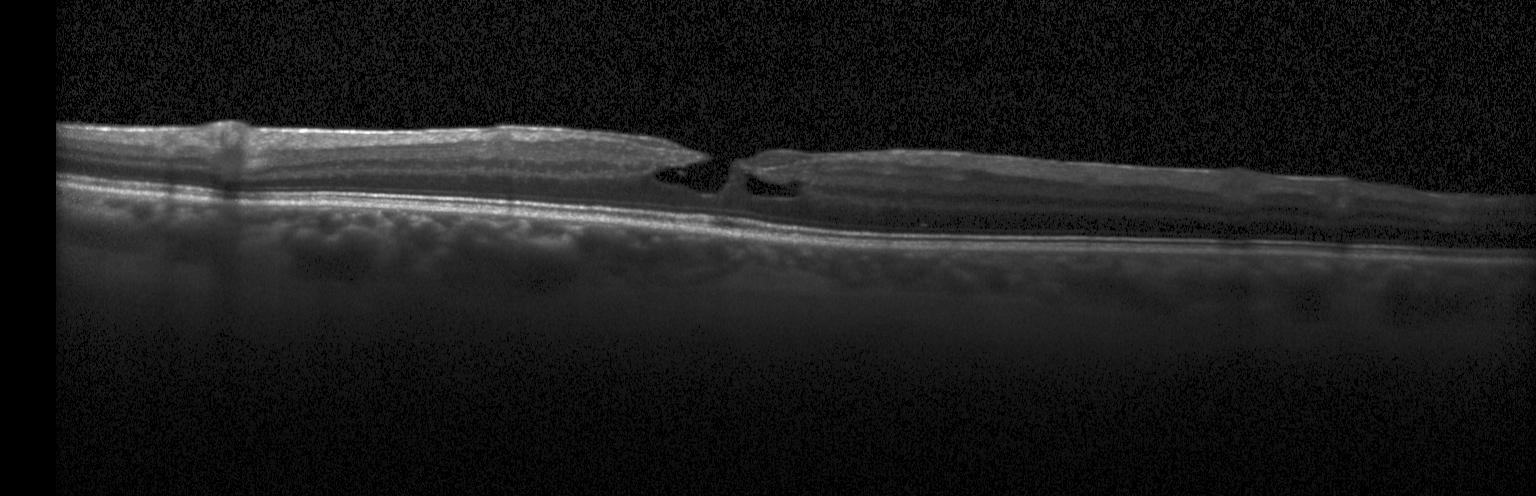

Optical coherence tomography scan · acquired on a Heidelberg Spectralis
Finding: diabetic macular edema (DME).